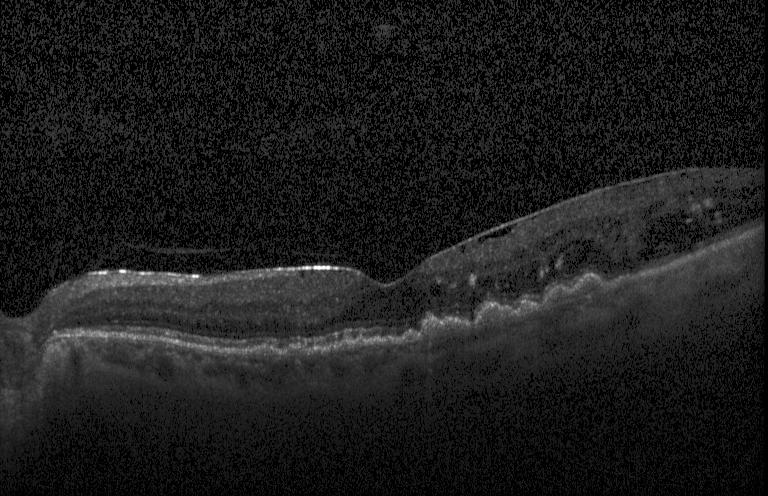

Retinal OCT B-scan. The scan shows drusen.